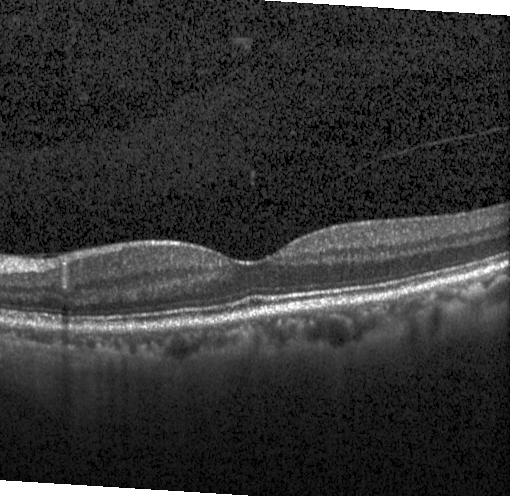
The scan shows no choroidal neovascularization, diabetic macular edema, or drusen.